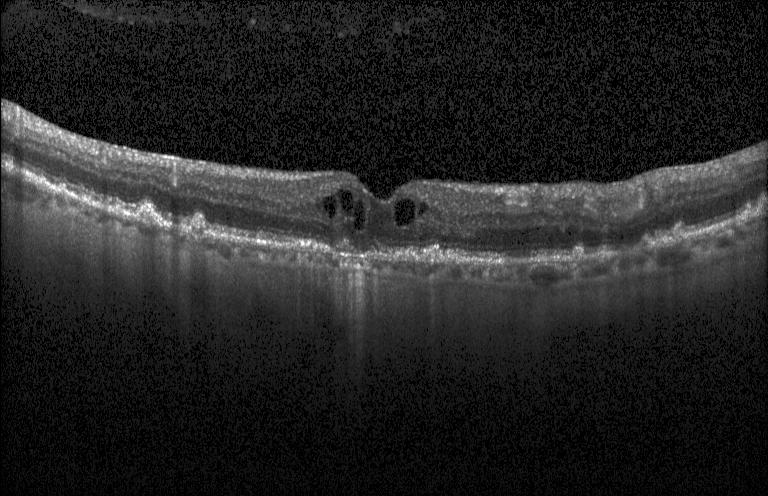
Instrument: Heidelberg Spectralis, retinal OCT cross-section, spectral-domain optical coherence tomography.
Finding: a choroidal neovascular membrane.